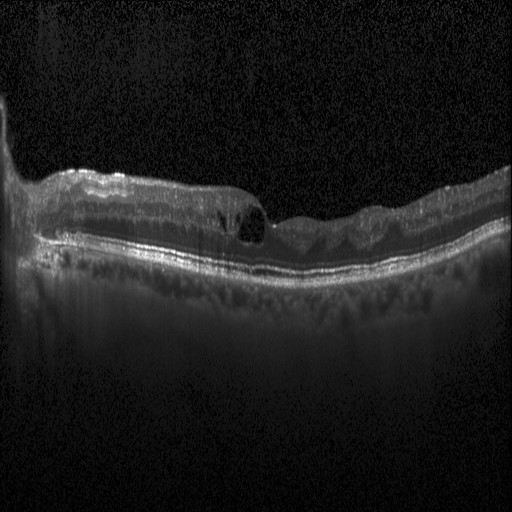
Finding: diabetic macular edema (DME).